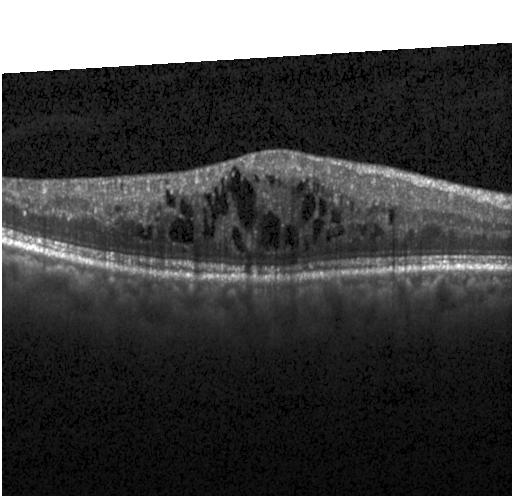

OCT B-scan. Macular scan. Acquired on a Heidelberg Spectralis.
OCT finding: diabetic macular edema.